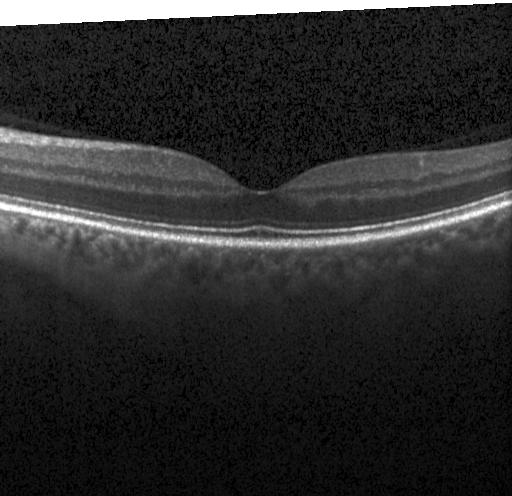

OCT line scan — Diagnosis: no choroidal neovascularization, no diabetic macular edema, and no drusen.